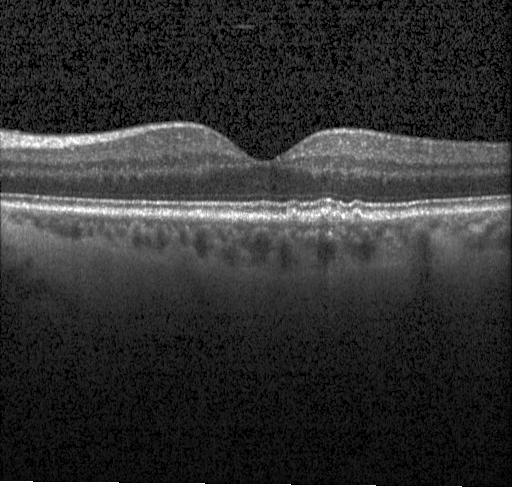

Centered on the fovea; Heidelberg Spectralis; SD-OCT; optical coherence tomography scan. Impression: sub-RPE drusenoid deposits.